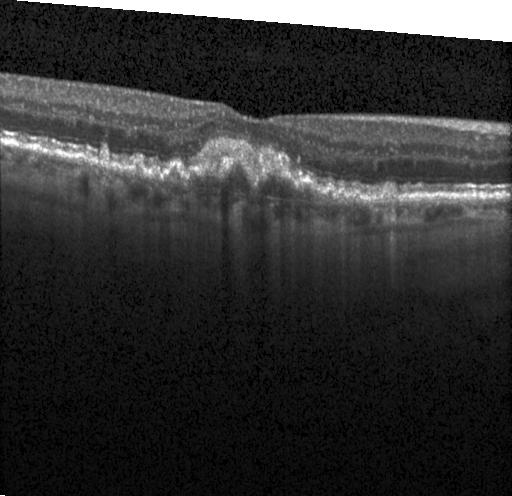

Retinal OCT B-scan; through the macula
A choroidal neovascular membrane.